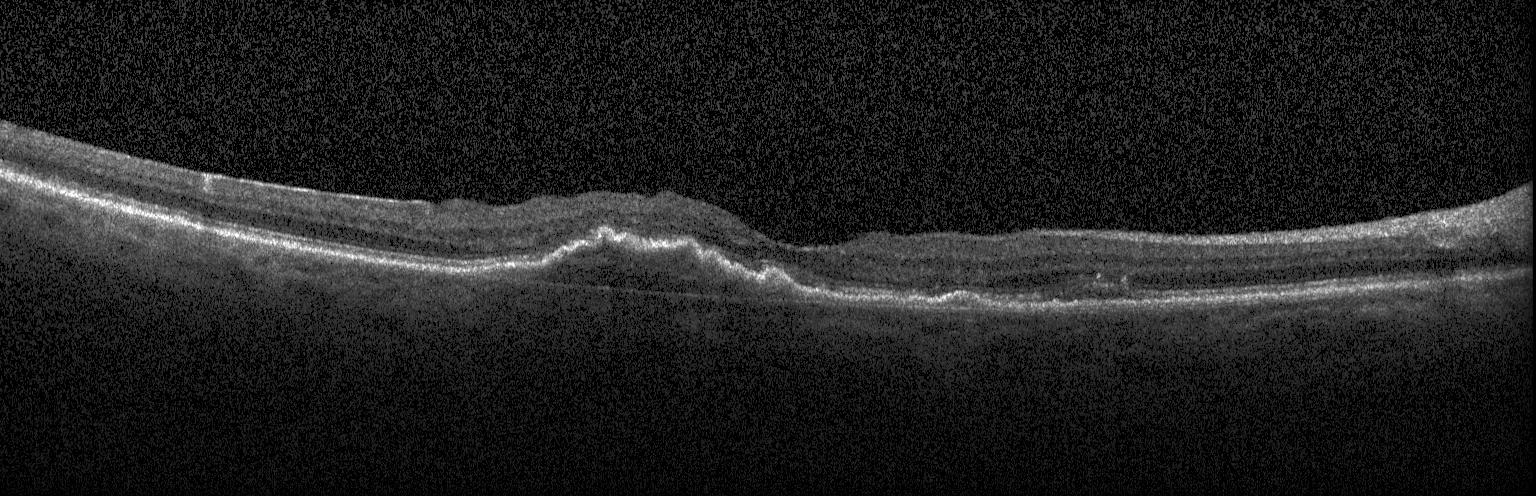 OCT finding: choroidal neovascularization.